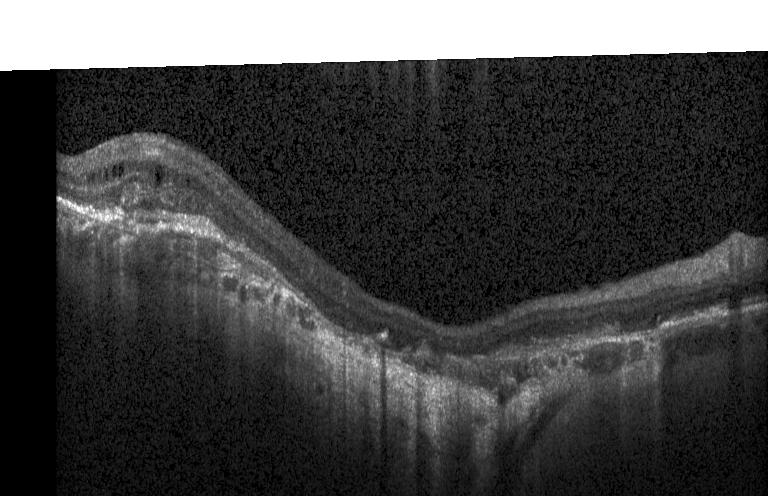

Macular OCT: a choroidal neovascular membrane.